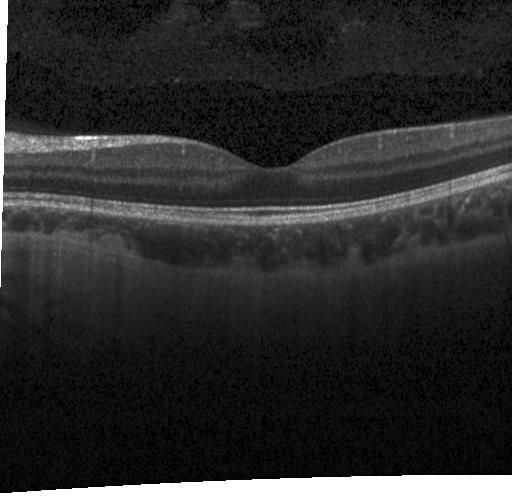

Macular OCT: no evidence of CNV, DME, or drusen.